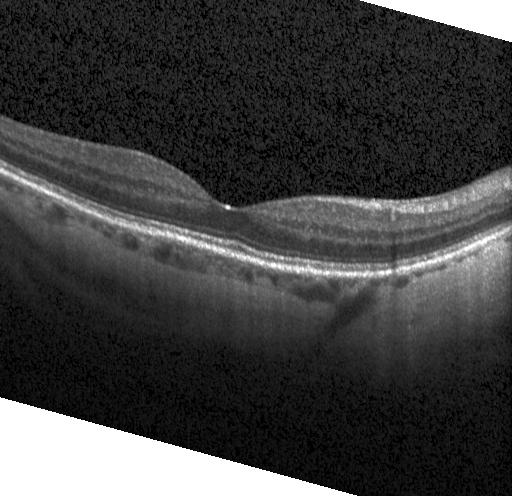
OCT B-scan showing neither CNV, DME, nor drusen.